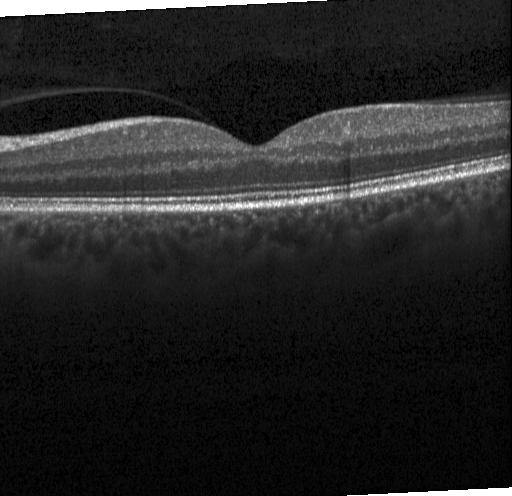

Through the macula; retinal OCT cross-section — Impression: no CNV, no DME, and no drusen.